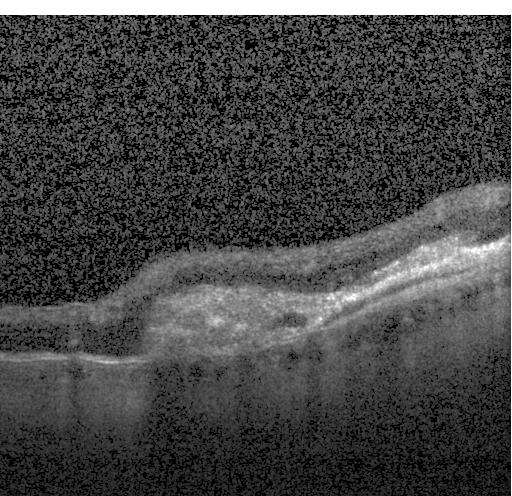 Through the macula; optical coherence tomography scan; SD-OCT — Diagnosis: a choroidal neovascular membrane.